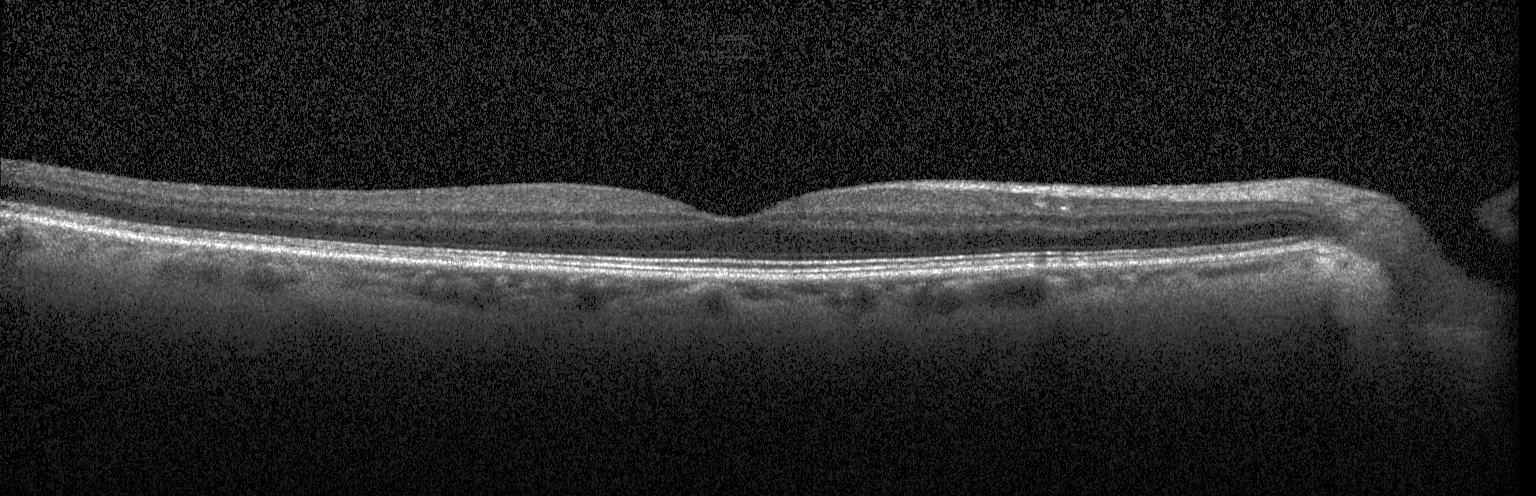

Retinal OCT cross-section · spectral-domain OCT.
Macular OCT: no CNV, DME, or drusen.